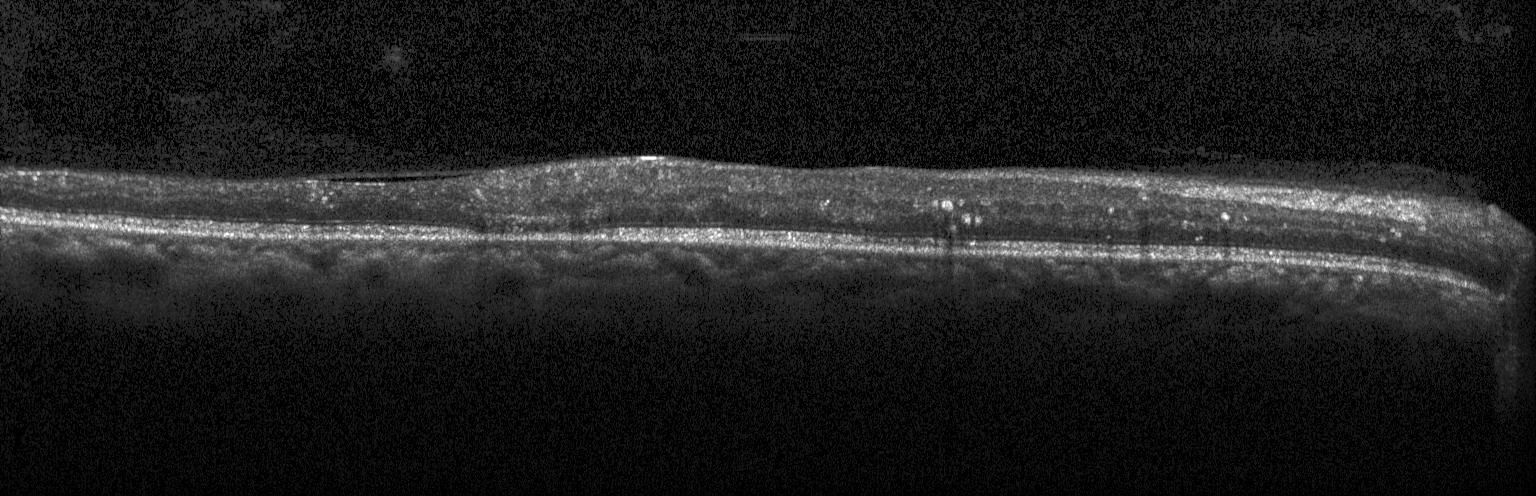
Acquired on a Heidelberg Spectralis, centered on the fovea, optical coherence tomography B-scan, spectral-domain OCT
Diabetic macular edema (DME).